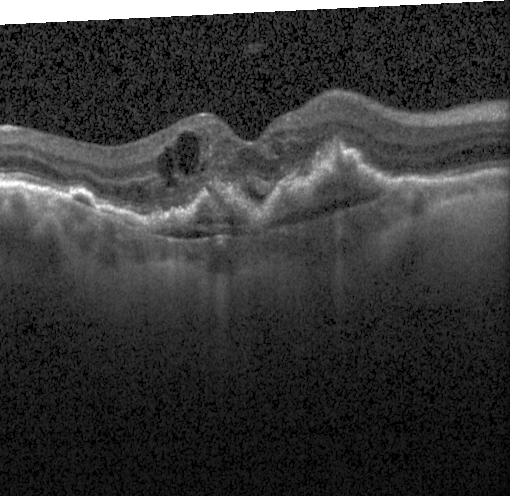 Retinal OCT B-scan. Assessment: a choroidal neovascular membrane.